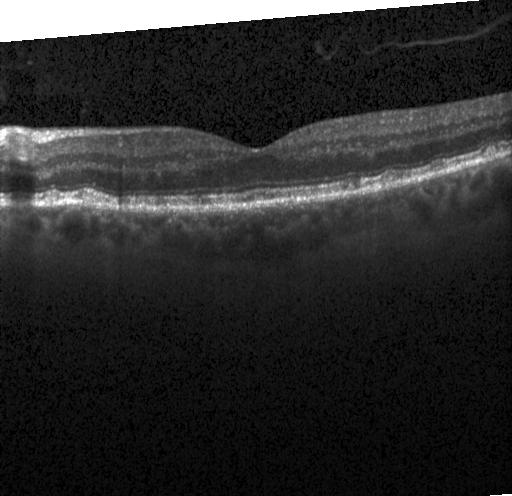 Fovea-centered, instrument: Heidelberg Spectralis, spectral-domain optical coherence tomography, retinal OCT cross-section — Macular OCT: multiple drusen.